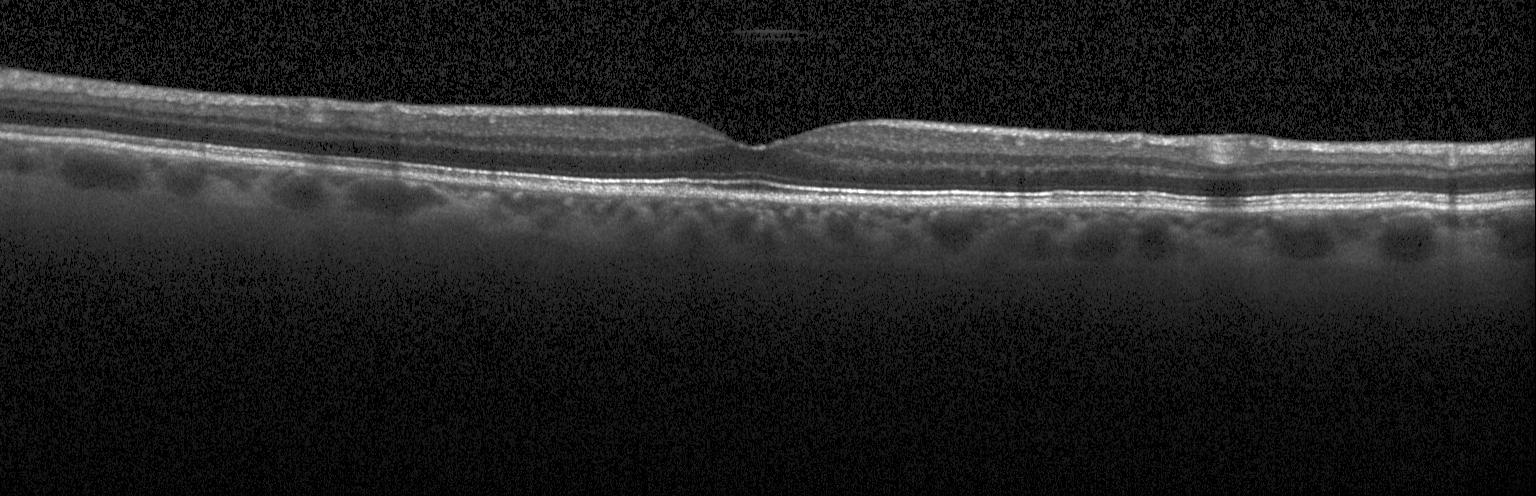 Heidelberg Spectralis, centered on the fovea, spectral-domain optical coherence tomography, optical coherence tomography B-scan. Finding: neither CNV, DME, nor drusen.